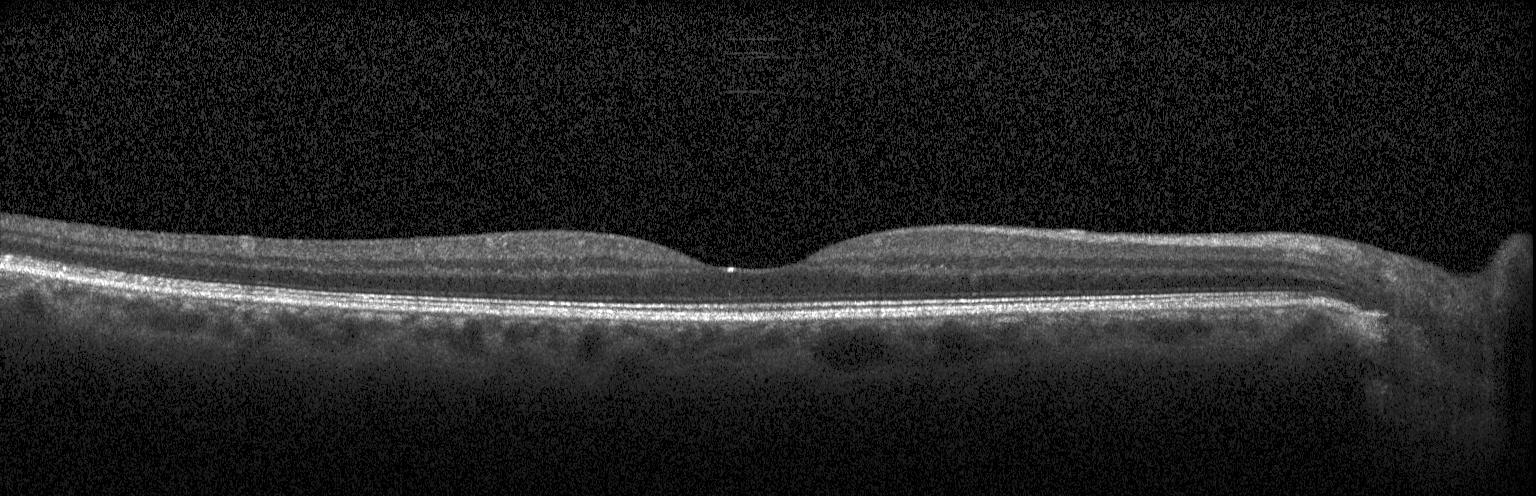 Diagnosis: no evidence of CNV, DME, or drusen.